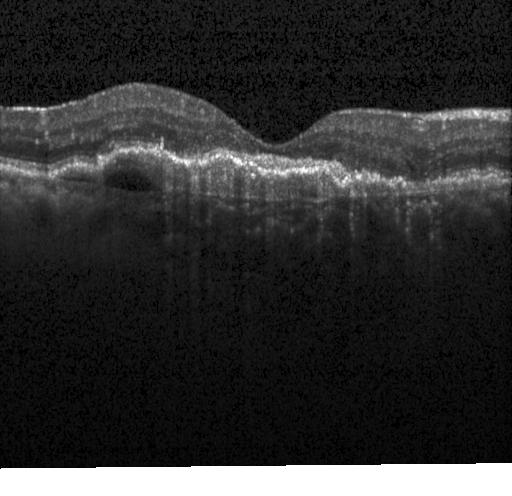

Diagnosis: CNV.